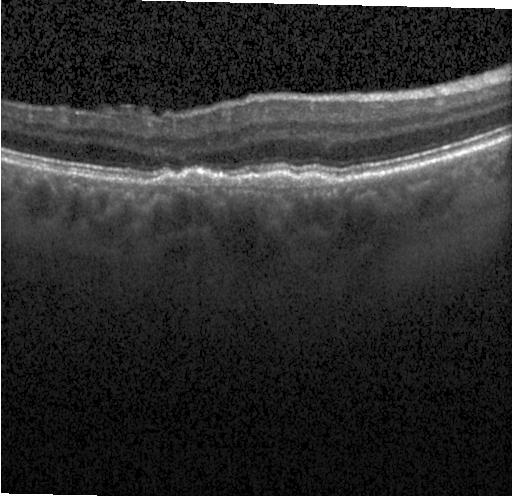

Assessment: a choroidal neovascular membrane.